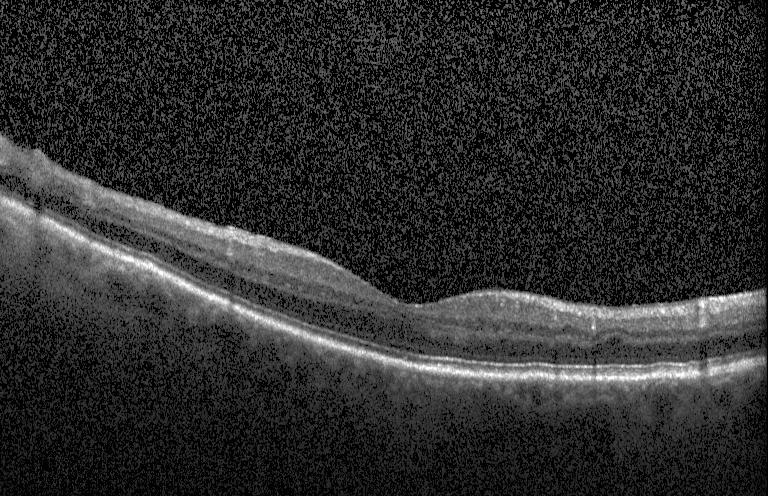
Diagnosis: neither CNV, DME, nor drusen.